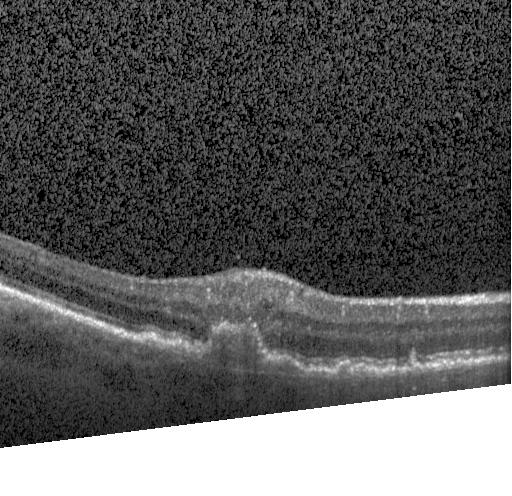
Spectral-domain OCT B-scan: choroidal neovascularization (CNV).